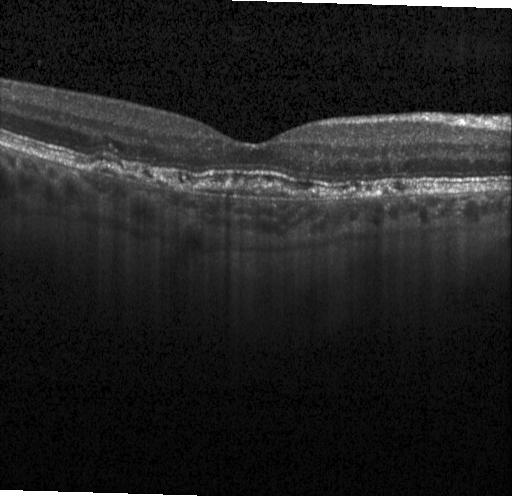 Heidelberg Spectralis OCT system. Retinal OCT B-scan. Macular scan. Spectral-domain OCT.
Finding: choroidal neovascularization.